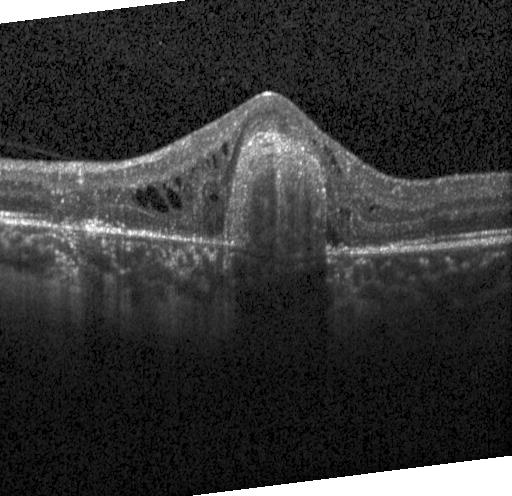
Retinal OCT B-scan
Assessment: a choroidal neovascular membrane.